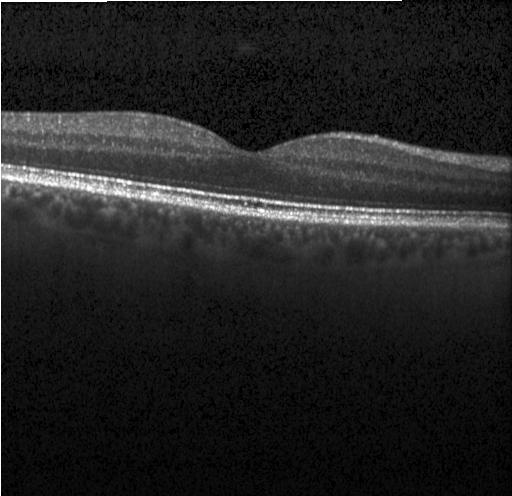

Diagnosis: no choroidal neovascularization, diabetic macular edema, or drusen.